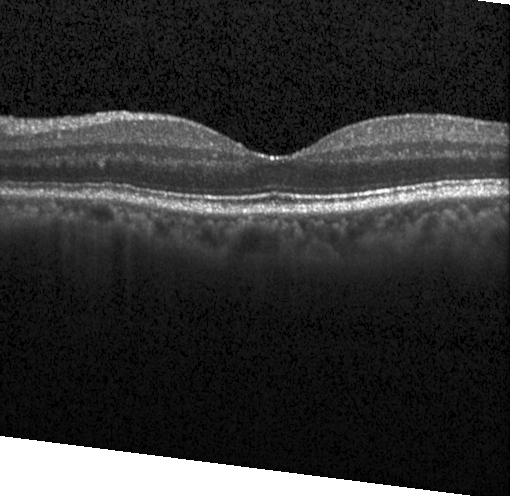 Centered on the fovea; OCT B-scan
The scan shows neither CNV, DME, nor drusen.